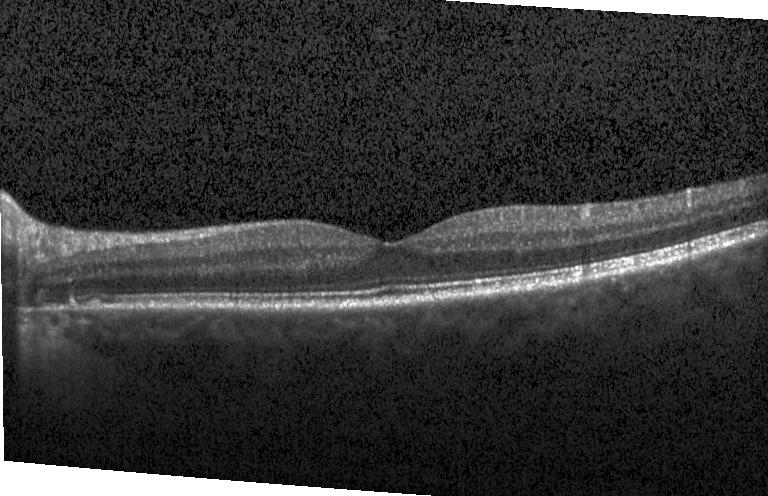
Macular scan; OCT line scan.
Macular OCT: no evidence of choroidal neovascularization, diabetic macular edema, or drusen.